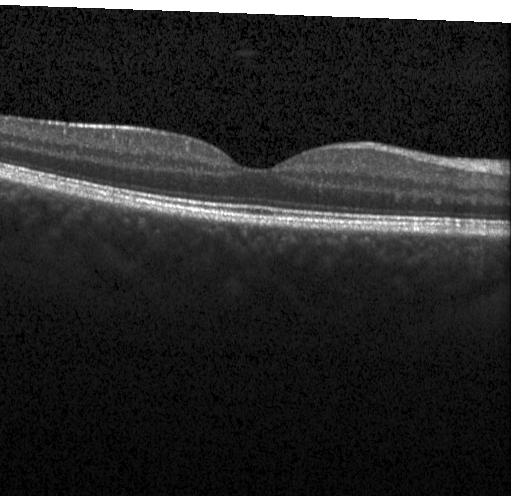 Acquired on a Heidelberg Spectralis. Spectral-domain optical coherence tomography. OCT B-scan. Dx: no choroidal neovascularization, no diabetic macular edema, and no drusen.